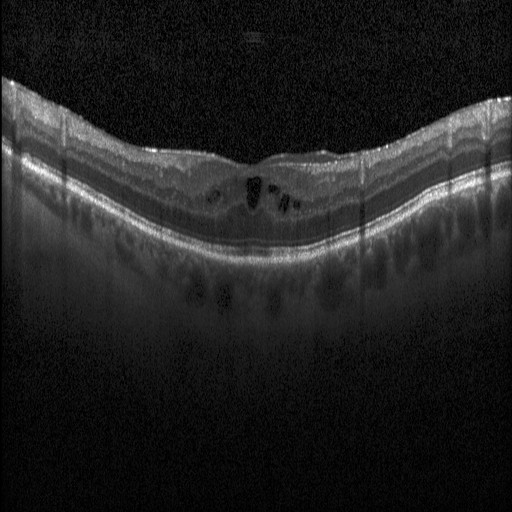 Diagnosis: DME.